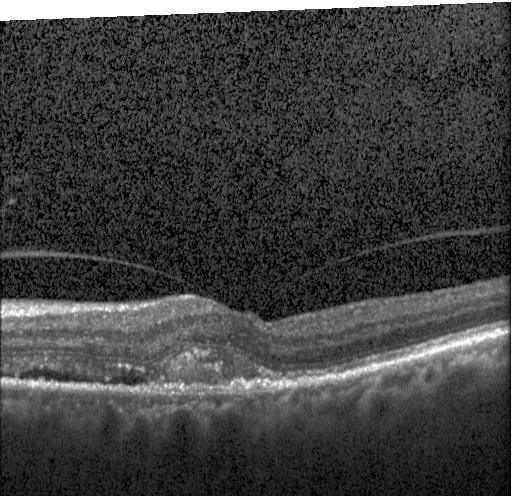
Dx: a choroidal neovascular membrane.